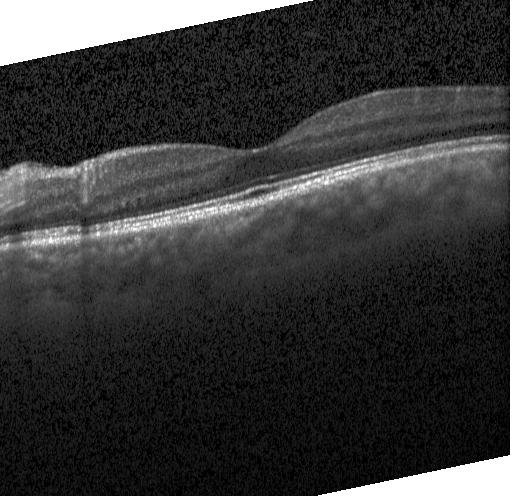 Optical coherence tomography B-scan
No choroidal neovascularization, diabetic macular edema, or drusen.